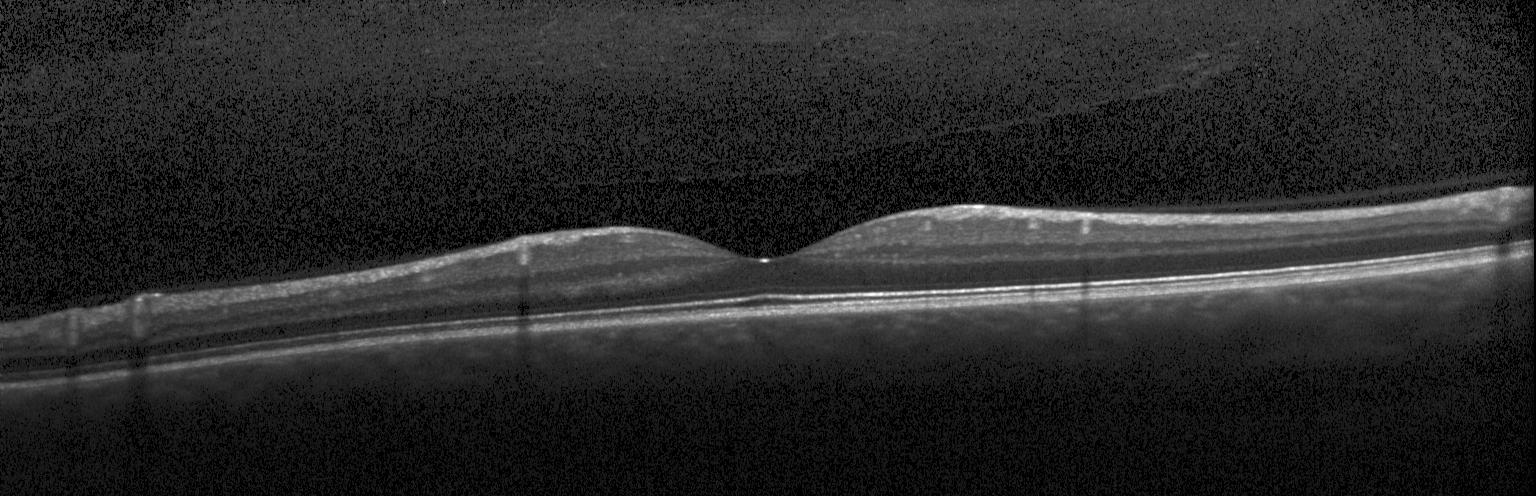 OCT B-scan, horizontal scan through the fovea, acquired on a Heidelberg Spectralis
Macular OCT: no choroidal neovascularization, no diabetic macular edema, and no drusen.